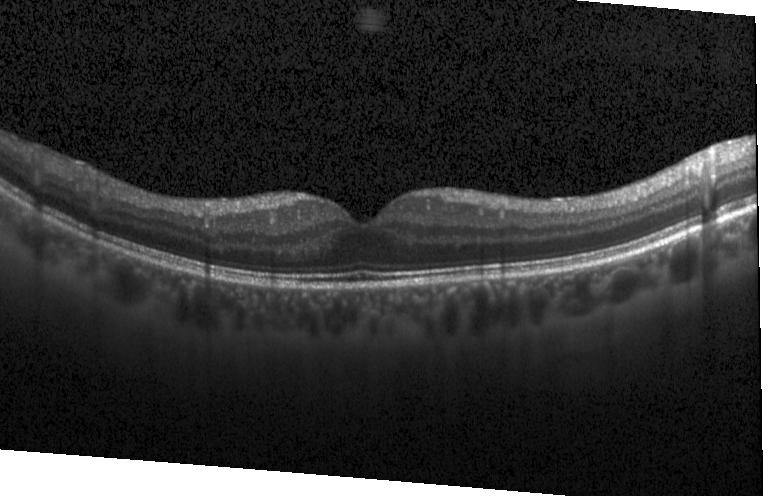

Heidelberg Spectralis · horizontal scan through the fovea · retinal OCT cross-section · SD-OCT.
Dx: no evidence of CNV, DME, or drusen.